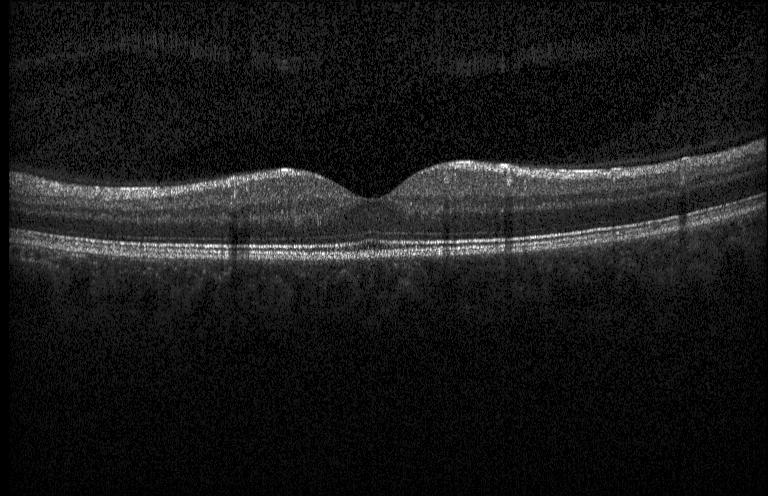

Heidelberg Spectralis OCT system · horizontal scan through the fovea · spectral-domain OCT · retinal OCT B-scan.
Finding: neither choroidal neovascularization, diabetic macular edema, nor drusen.